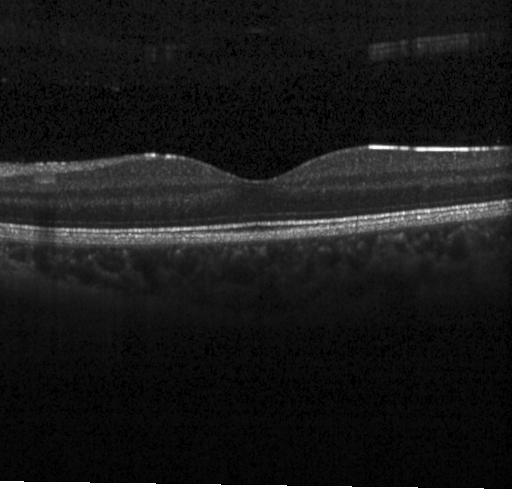 Heidelberg Spectralis, spectral-domain optical coherence tomography, retinal OCT B-scan — Neither choroidal neovascularization, diabetic macular edema, nor drusen.